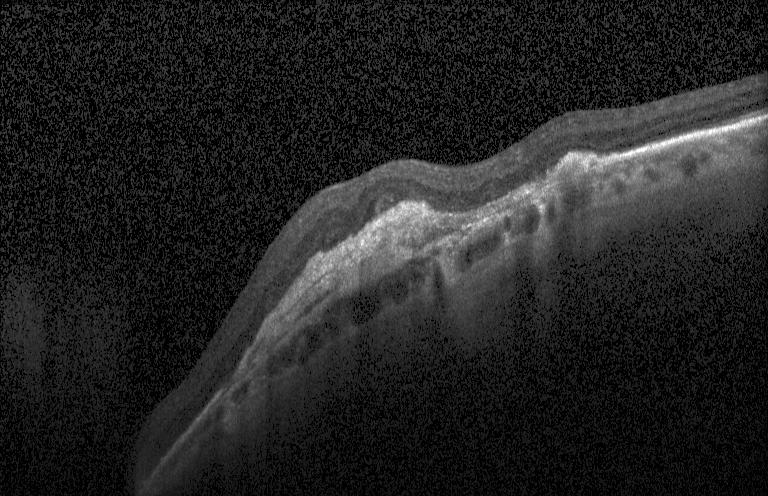
Choroidal neovascularization (CNV).